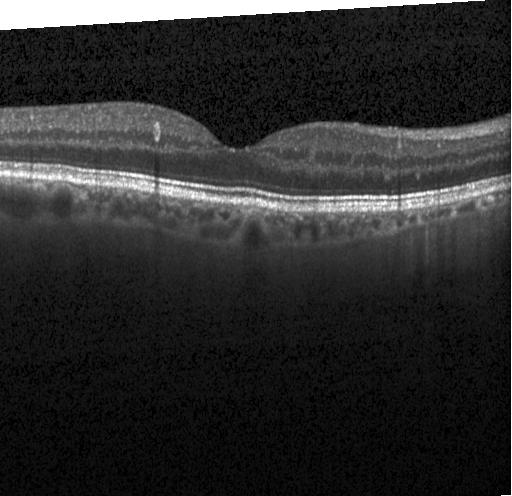

OCT B-scan, centered on the fovea — Macular OCT: no choroidal neovascularization, no diabetic macular edema, and no drusen.